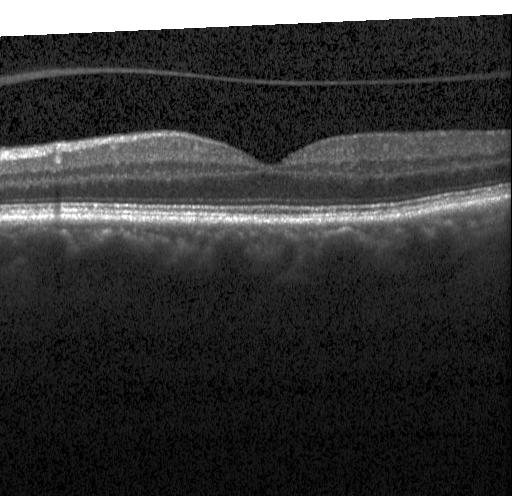
No choroidal neovascularization, no diabetic macular edema, and no drusen.